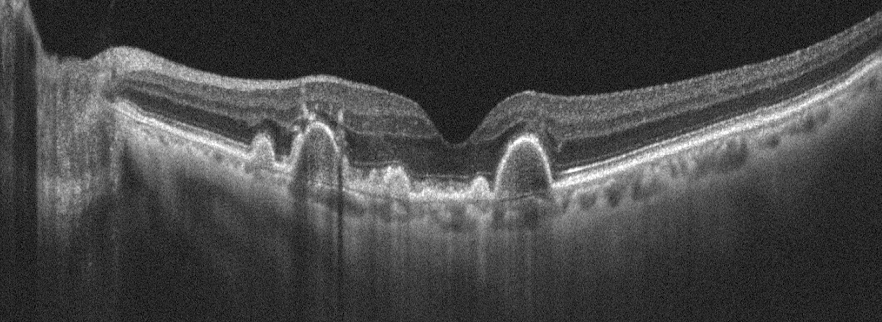 Optical coherence tomography scan; oculus sinister — Age-related macular degeneration.